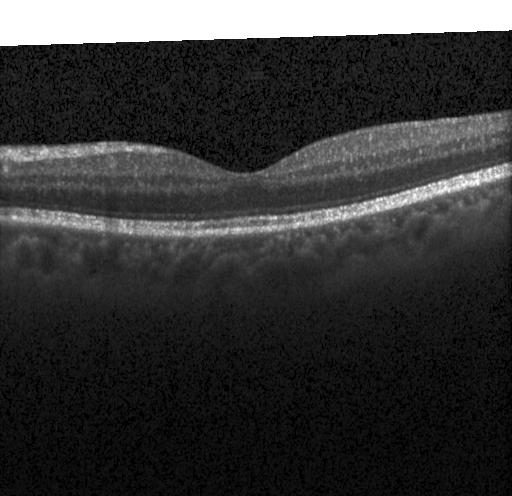
OCT B-scan; instrument: Heidelberg Spectralis; fovea-centered — Impression: no choroidal neovascularization, diabetic macular edema, or drusen.